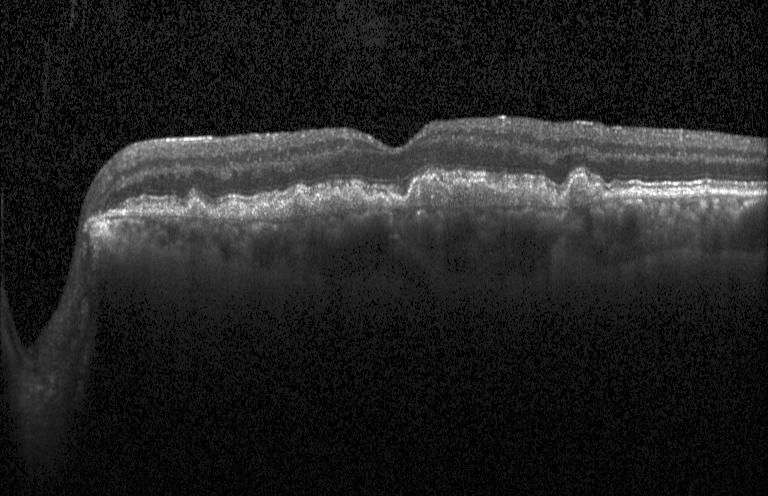 OCT B-scan showing CNV.